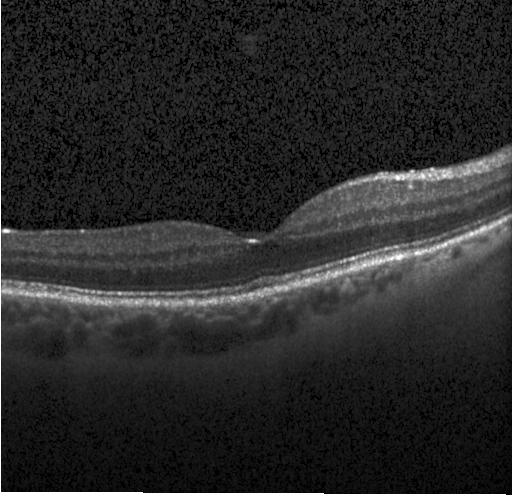

SD-OCT. Horizontal scan through the fovea. OCT line scan. Instrument: Heidelberg Spectralis.
Diagnosis: no choroidal neovascularization, no diabetic macular edema, and no drusen.